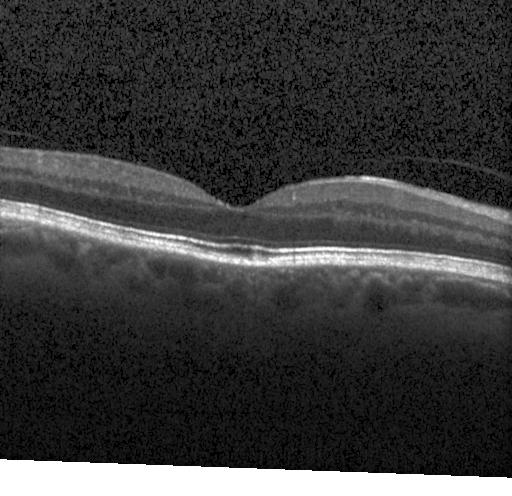 Spectral-domain optical coherence tomography, optical coherence tomography scan, instrument: Heidelberg Spectralis, fovea-centered. Impression: no choroidal neovascularization, no diabetic macular edema, and no drusen.